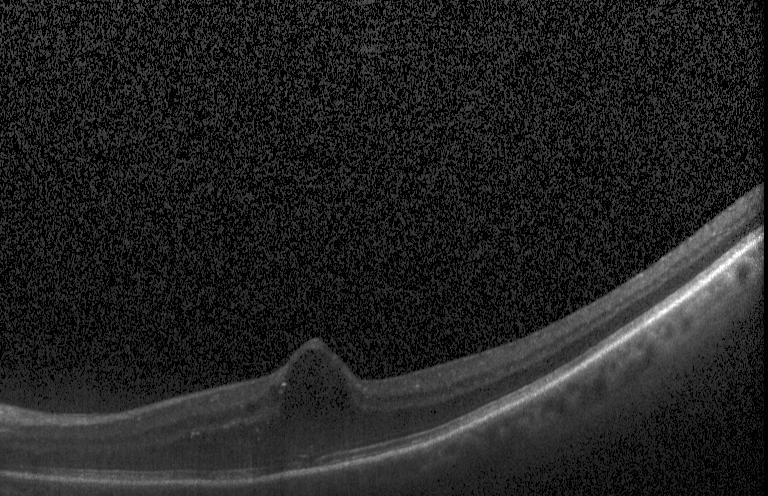

Optical coherence tomography B-scan
Dx: diabetic macular edema (DME).